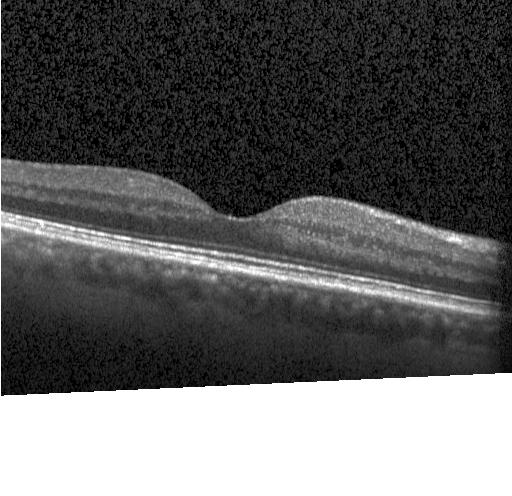 Optical coherence tomography B-scan. Diagnosis: no CNV, no DME, and no drusen.